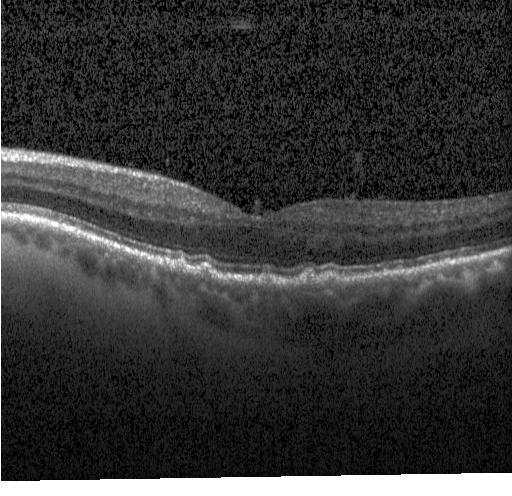 Heidelberg Spectralis OCT system · OCT B-scan
The scan shows drusen.